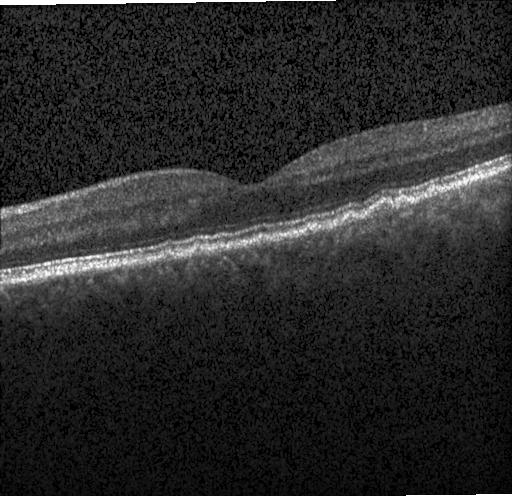

Retinal OCT B-scan
Finding: multiple drusen.